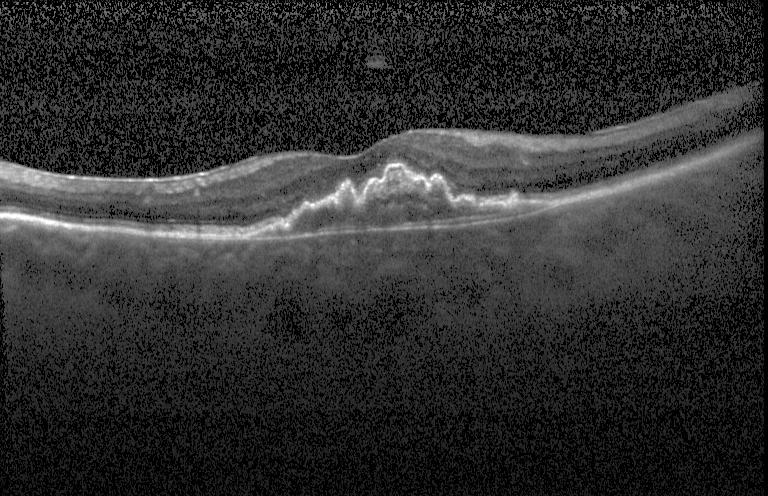 Retinal OCT cross-section. Macular scan. Spectral-domain OCT. Acquired on a Heidelberg Spectralis. The scan shows choroidal neovascularization (CNV).